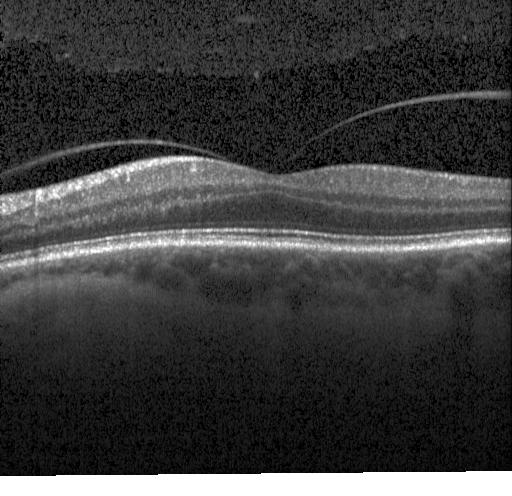

Optical coherence tomography scan
The scan shows no evidence of CNV, DME, or drusen.